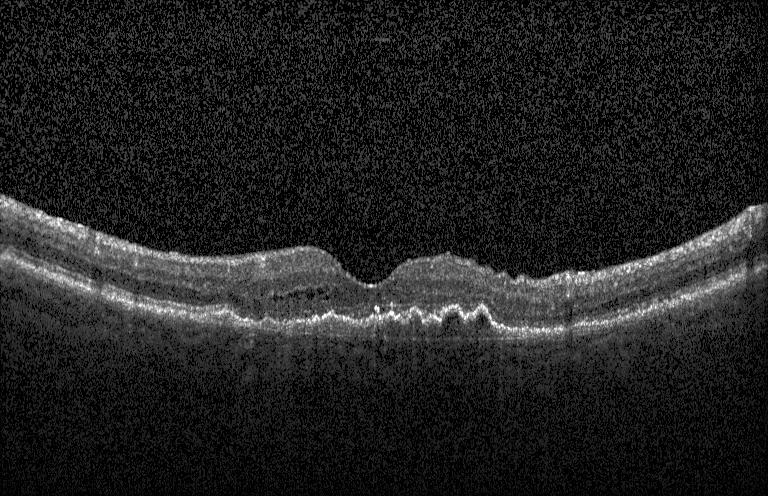

OCT line scan
The scan shows a choroidal neovascular membrane.